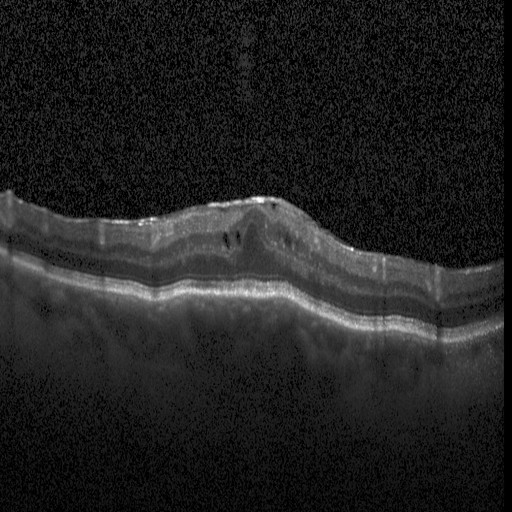 Acquired on a Heidelberg Spectralis; optical coherence tomography B-scan; centered on the fovea; spectral-domain OCT — Finding: DME.